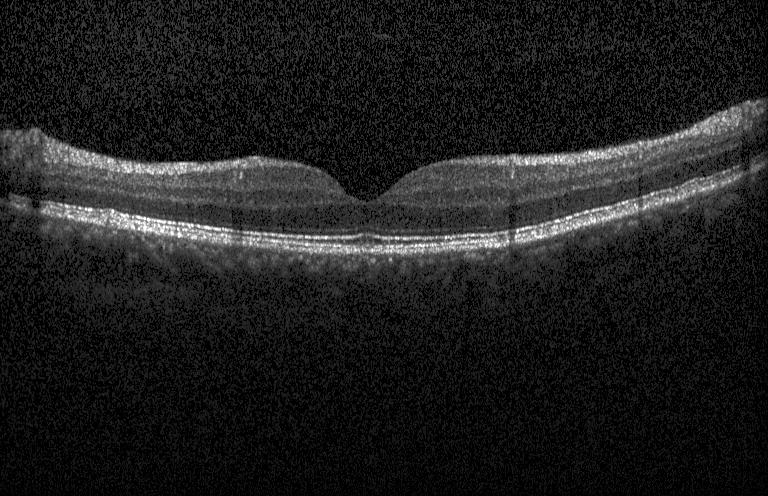
The scan shows neither CNV, DME, nor drusen.